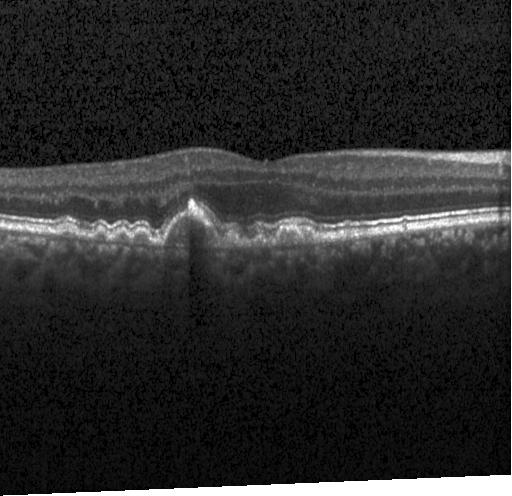
Optical coherence tomography B-scan. Horizontal scan through the fovea. Finding: multiple drusen.